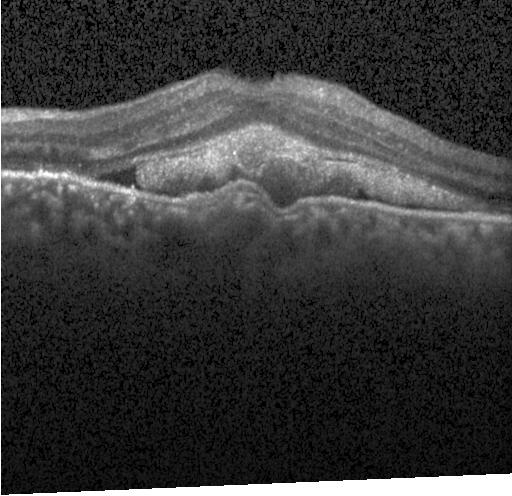 Macular OCT demonstrating a choroidal neovascular membrane.